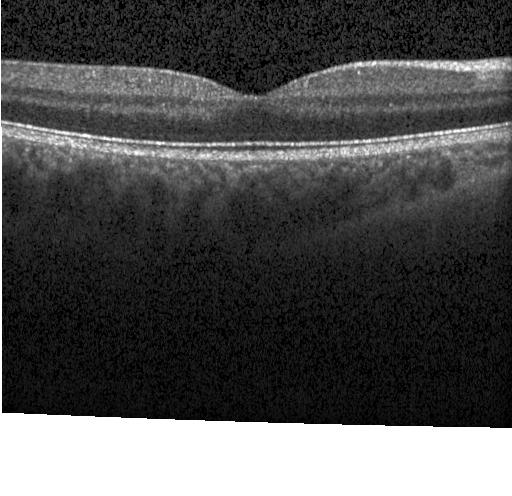 Macular OCT demonstrating no choroidal neovascularization, no diabetic macular edema, and no drusen.